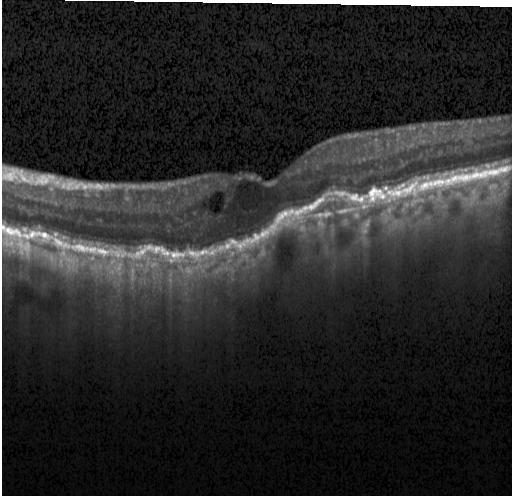
Diagnosis: a choroidal neovascular membrane.